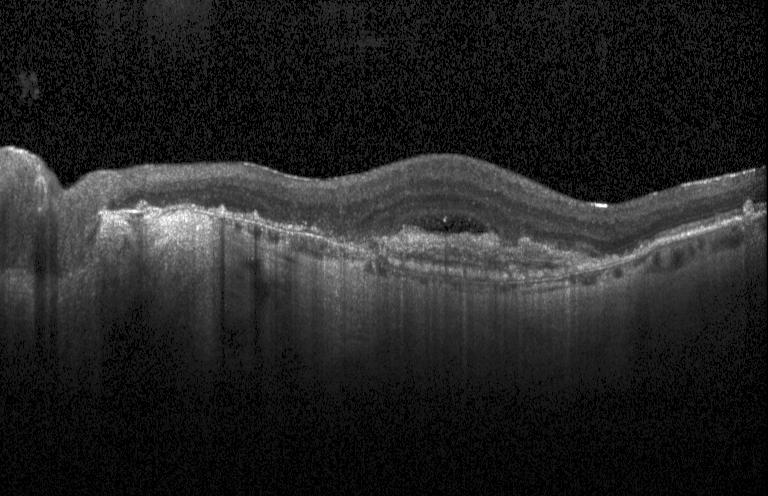 A choroidal neovascular membrane.